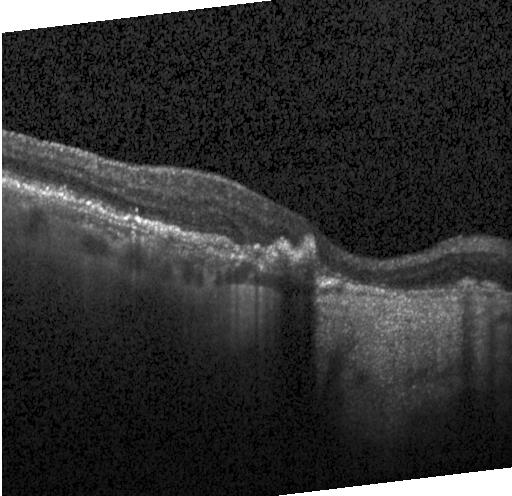

OCT finding: a choroidal neovascular membrane.